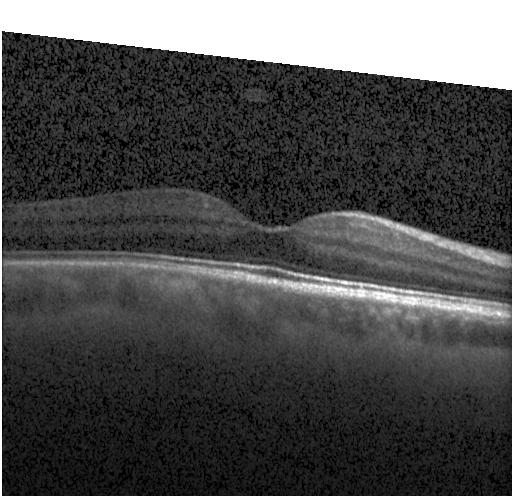

OCT B-scan
Impression: neither choroidal neovascularization, diabetic macular edema, nor drusen.